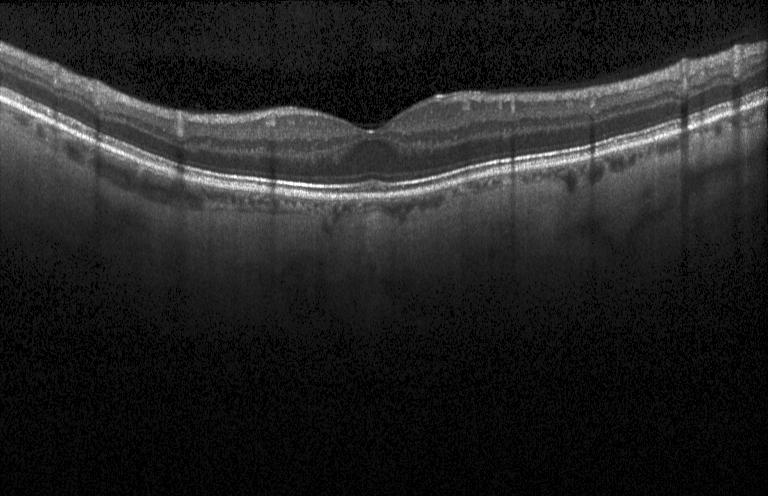
Impression: no choroidal neovascularization, no diabetic macular edema, and no drusen.